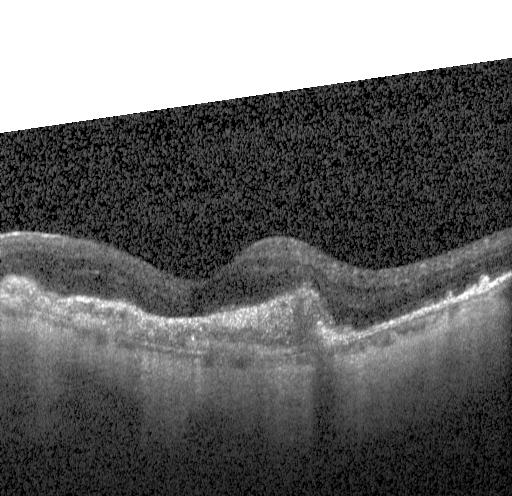

The scan shows choroidal neovascularization.